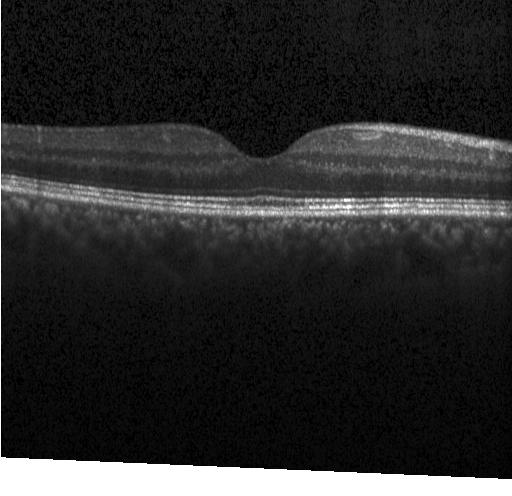

Spectral-domain OCT B-scan: no choroidal neovascularization, no diabetic macular edema, and no drusen.